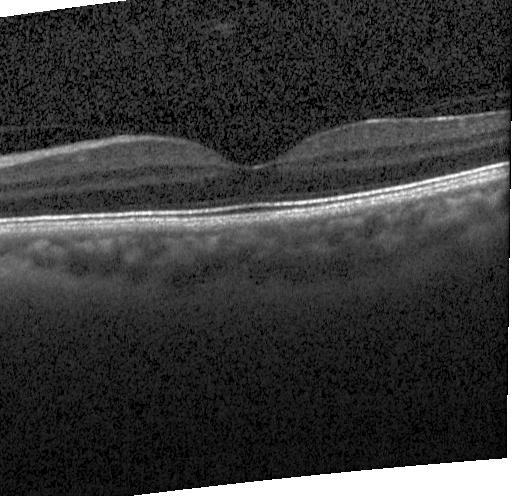 OCT B-scan showing no evidence of CNV, DME, or drusen.